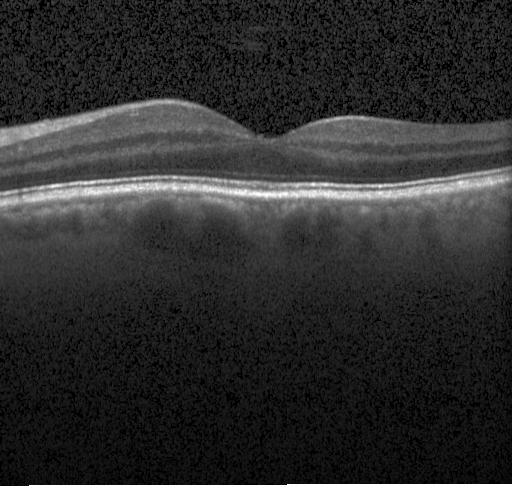 Finding: no CNV, no DME, and no drusen.